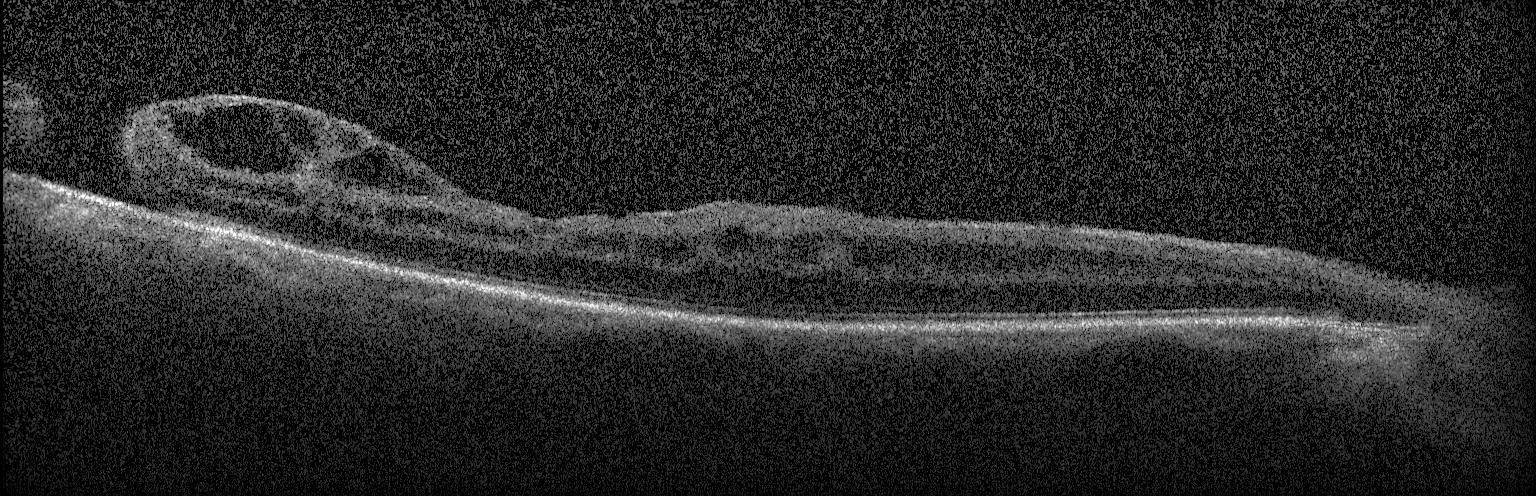 Macular OCT demonstrating DME.